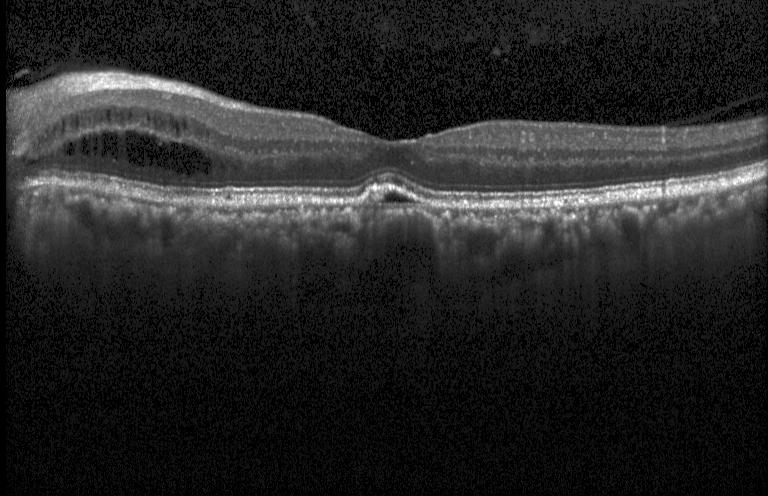
Finding: a choroidal neovascular membrane.